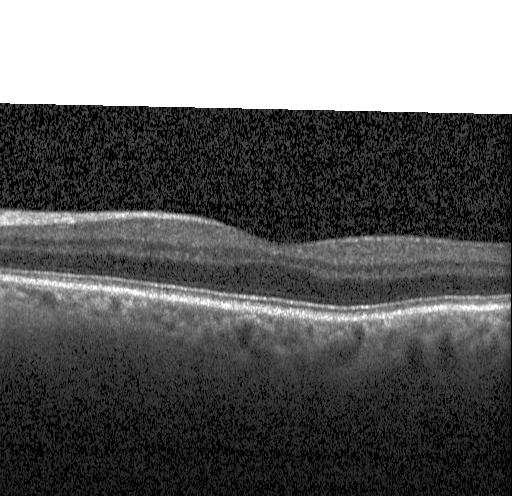

Finding: no evidence of choroidal neovascularization, diabetic macular edema, or drusen.